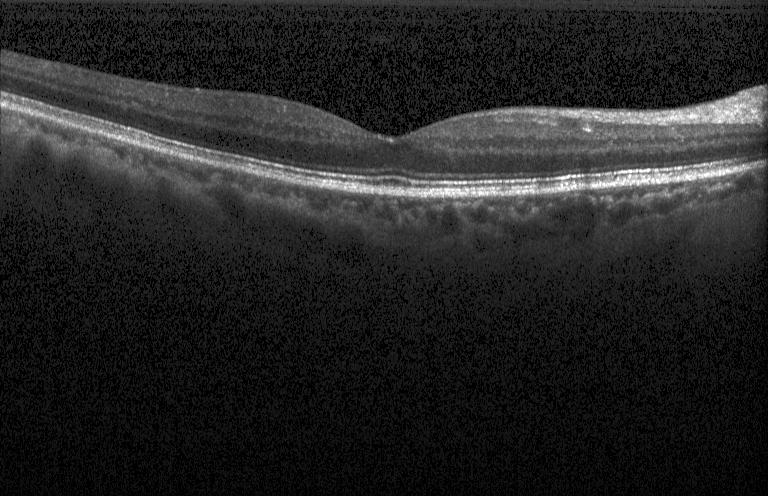

OCT line scan.
Impression: neither choroidal neovascularization, diabetic macular edema, nor drusen.